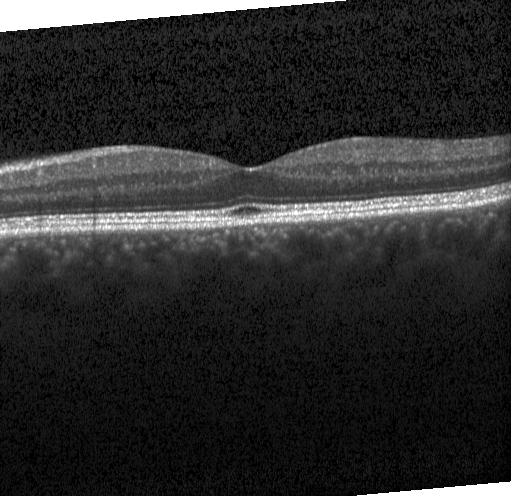

Retinal OCT B-scan. Assessment: neither choroidal neovascularization, diabetic macular edema, nor drusen.